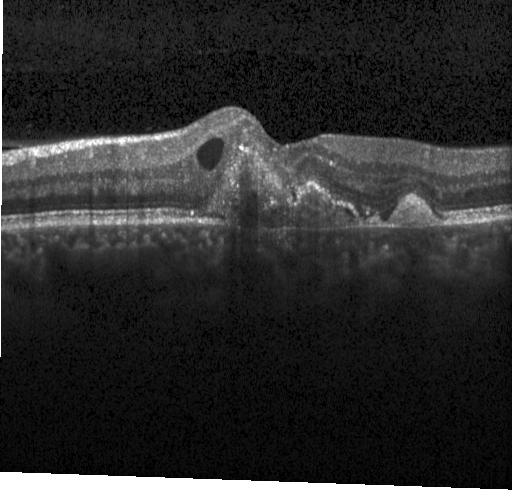 Retinal OCT B-scan, horizontal scan through the fovea, Heidelberg Spectralis OCT system. This B-scan demonstrates choroidal neovascularization.